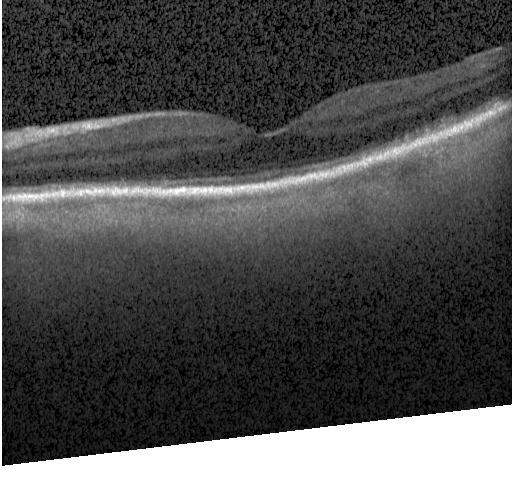

Finding: no choroidal neovascularization, no diabetic macular edema, and no drusen.